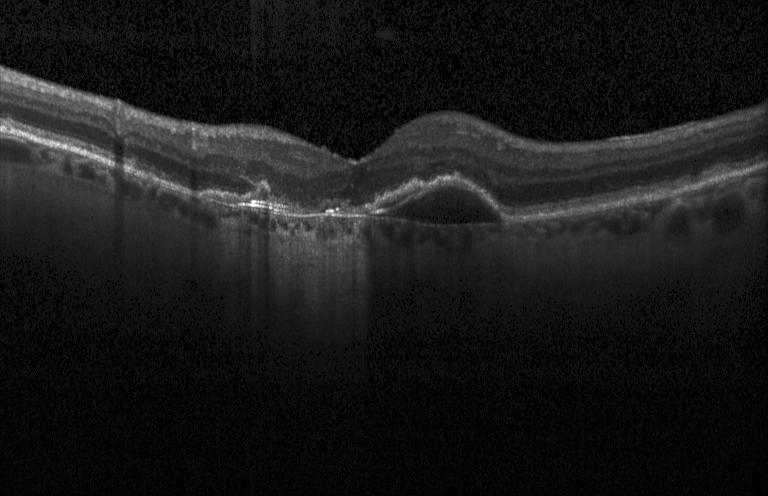

Through the macula, spectral-domain OCT, retinal OCT cross-section
Assessment: a choroidal neovascular membrane.